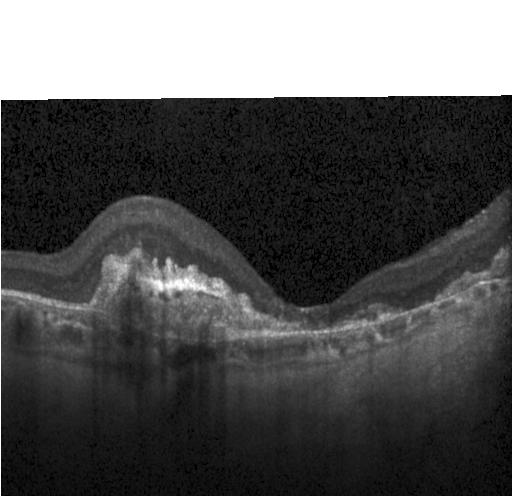 Optical coherence tomography scan. Acquired on a Heidelberg Spectralis
Finding: a choroidal neovascular membrane.